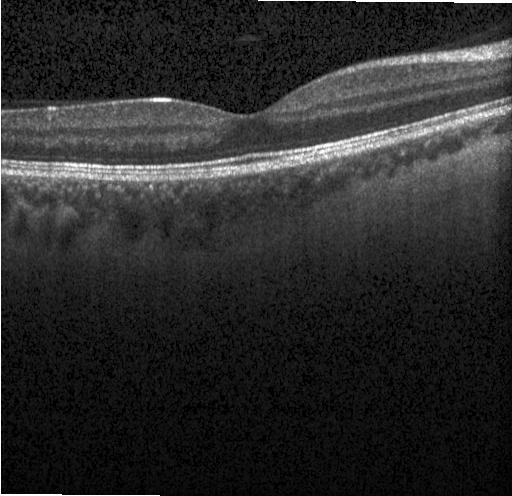

Spectral-domain OCT. Optical coherence tomography B-scan. Horizontal scan through the fovea. No choroidal neovascularization, no diabetic macular edema, and no drusen.